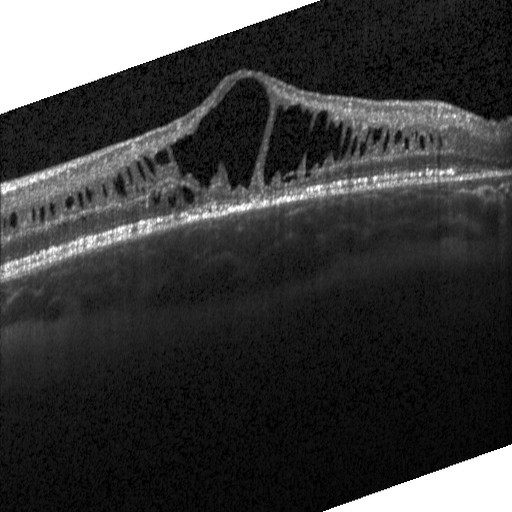
Spectral-domain OCT. Retinal OCT cross-section. Heidelberg Spectralis.
Finding: diabetic macular edema.